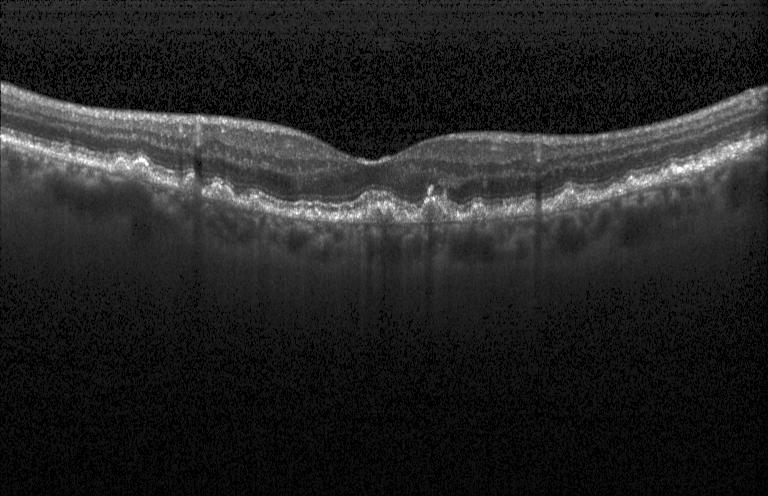 Drusen.